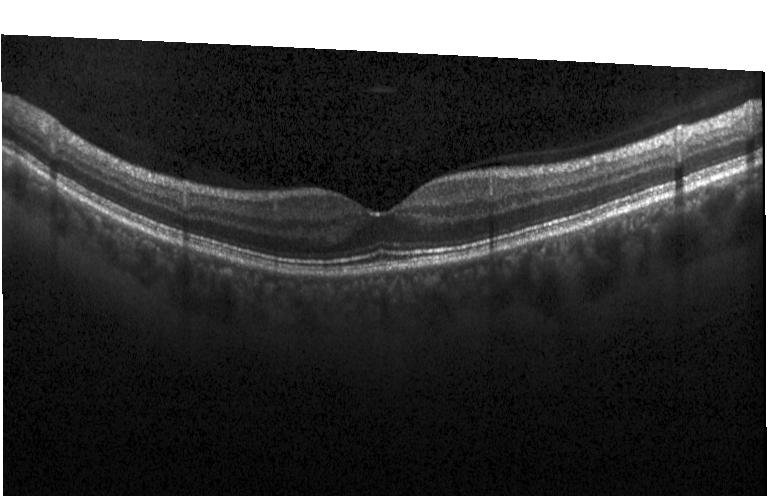

Impression: neither choroidal neovascularization, diabetic macular edema, nor drusen.